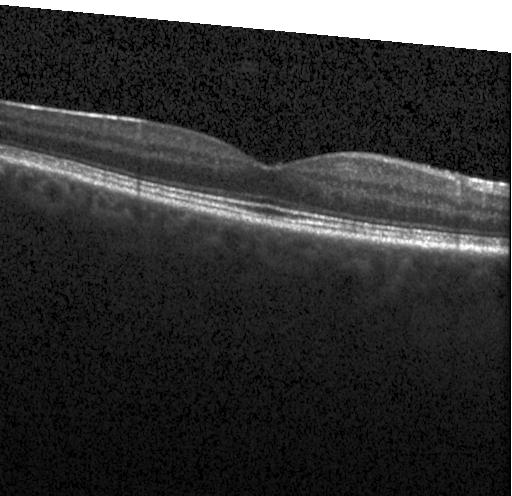
Instrument: Heidelberg Spectralis, optical coherence tomography scan — This B-scan demonstrates no choroidal neovascularization, diabetic macular edema, or drusen.